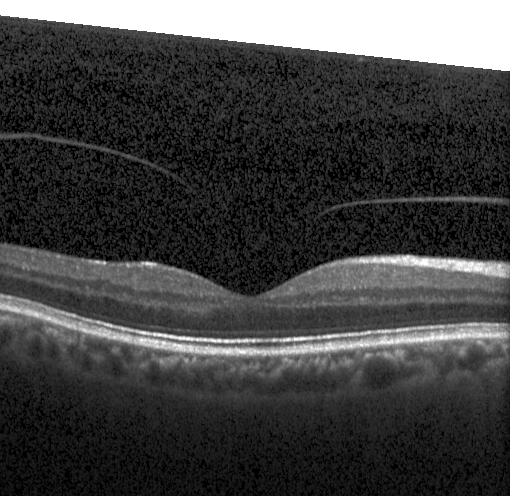
Retinal OCT cross-section — Diagnosis: no evidence of choroidal neovascularization, diabetic macular edema, or drusen.